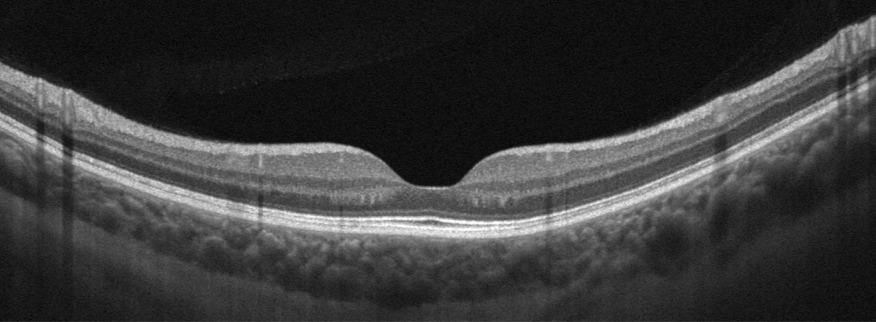
Diagnosis: no evidence of AMD, DME, ERM, RAO, RVO, or VID.